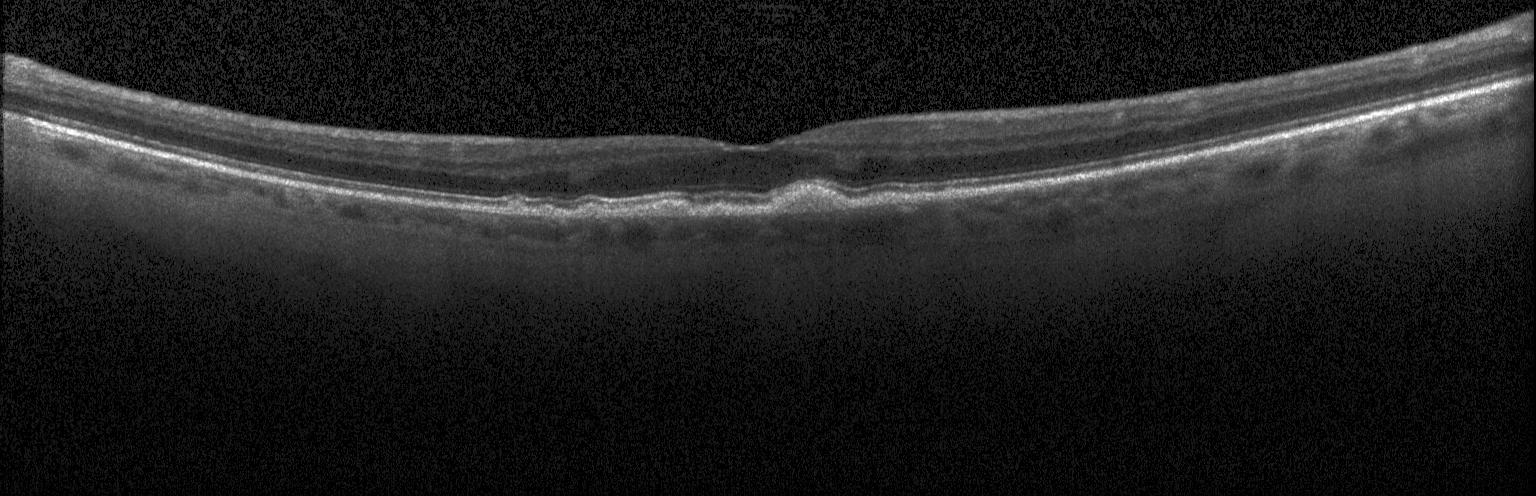

OCT scan showing drusen.